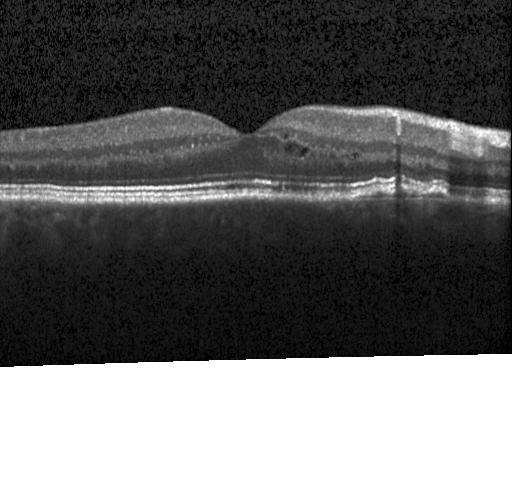 Heidelberg Spectralis OCT system; macular scan; spectral-domain OCT; optical coherence tomography scan — The scan shows a choroidal neovascular membrane.